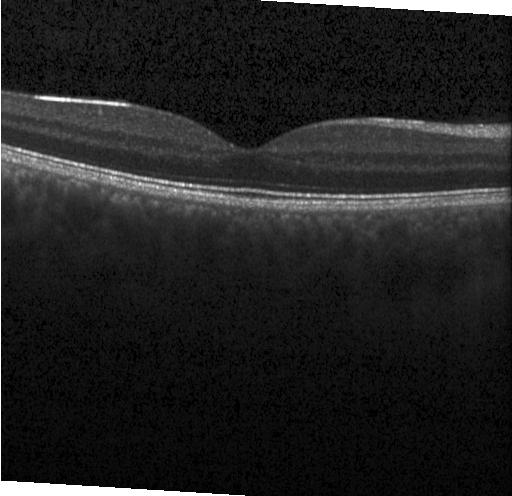
Optical coherence tomography B-scan — Impression: no choroidal neovascularization, no diabetic macular edema, and no drusen.